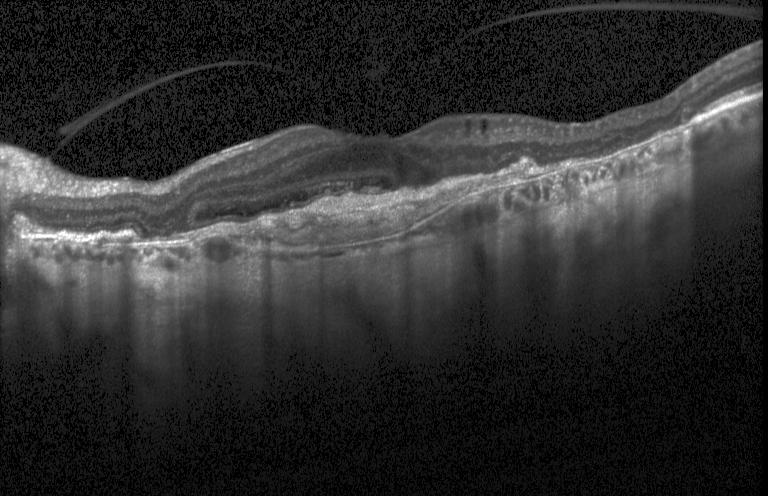 Retinal OCT B-scan; Heidelberg Spectralis
This B-scan demonstrates a choroidal neovascular membrane.